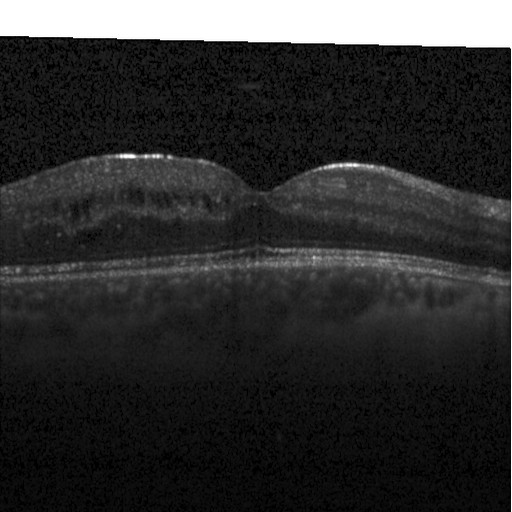

OCT finding: DME.